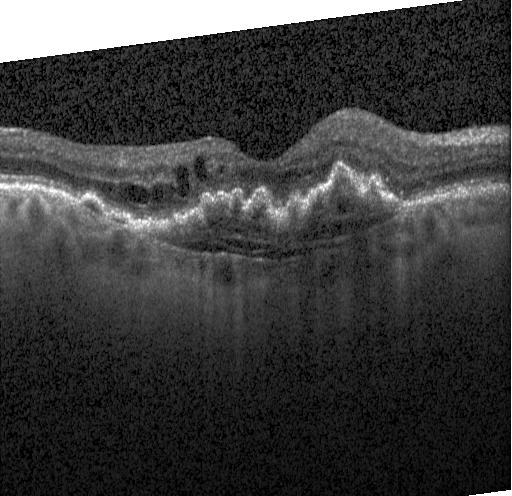
Macular scan; spectral-domain optical coherence tomography; Heidelberg Spectralis; retinal OCT cross-section.
Impression: a choroidal neovascular membrane.